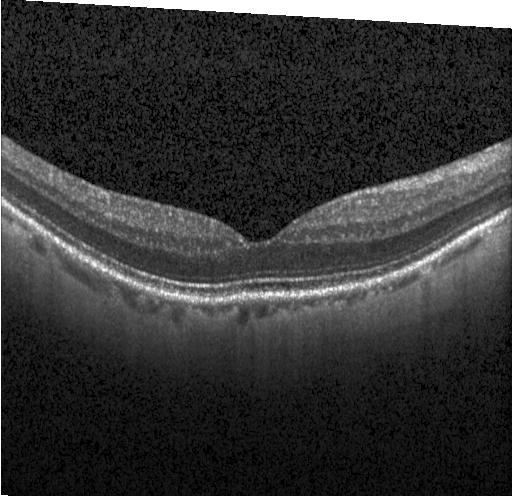
Instrument: Heidelberg Spectralis, spectral-domain optical coherence tomography, fovea-centered, OCT B-scan
Diagnosis: no evidence of CNV, DME, or drusen.